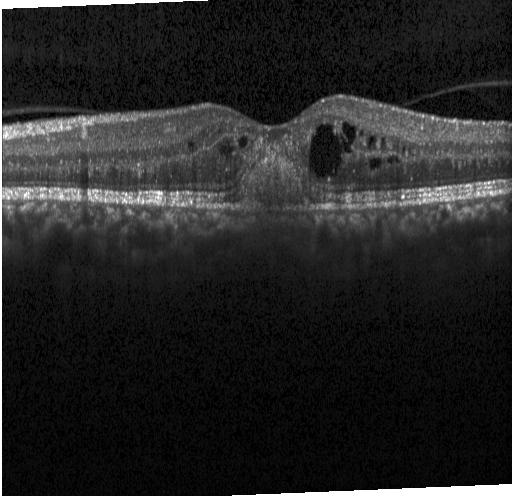 Retinal OCT cross-section showing CNV.